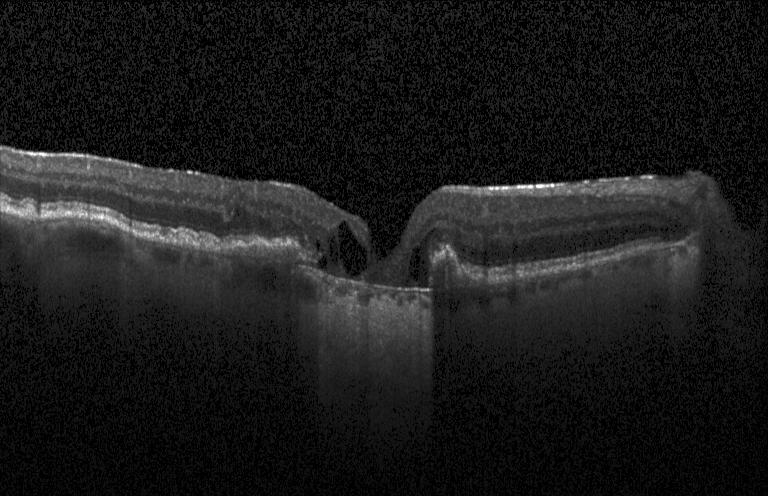 Heidelberg Spectralis OCT system · optical coherence tomography scan · horizontal scan through the fovea
The scan shows a choroidal neovascular membrane.